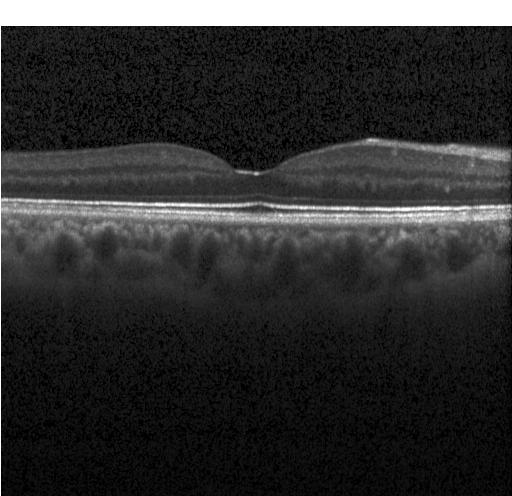 Spectral-domain OCT. Retinal OCT B-scan. Diagnosis: no evidence of choroidal neovascularization, diabetic macular edema, or drusen.